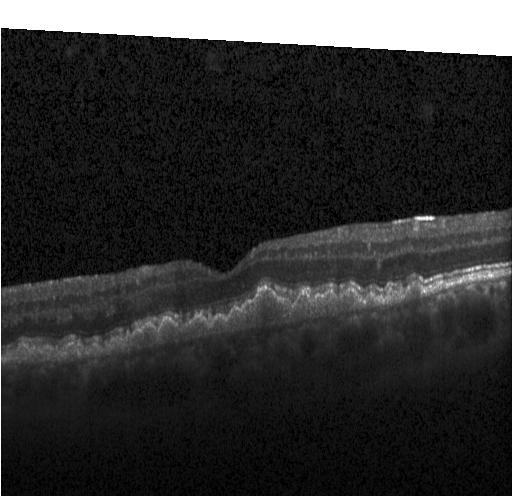 Dx: a choroidal neovascular membrane.